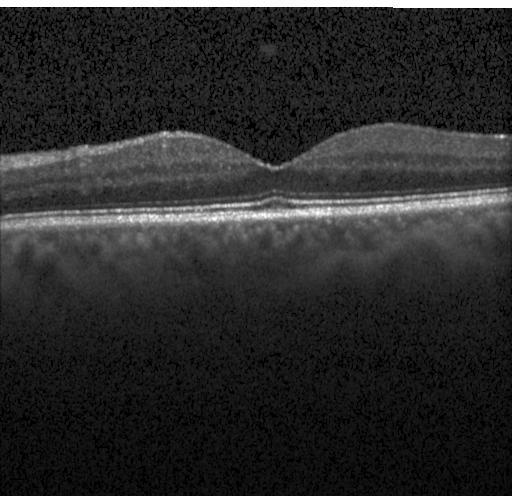 Retinal OCT cross-section, spectral-domain optical coherence tomography.
The scan shows no CNV, no DME, and no drusen.